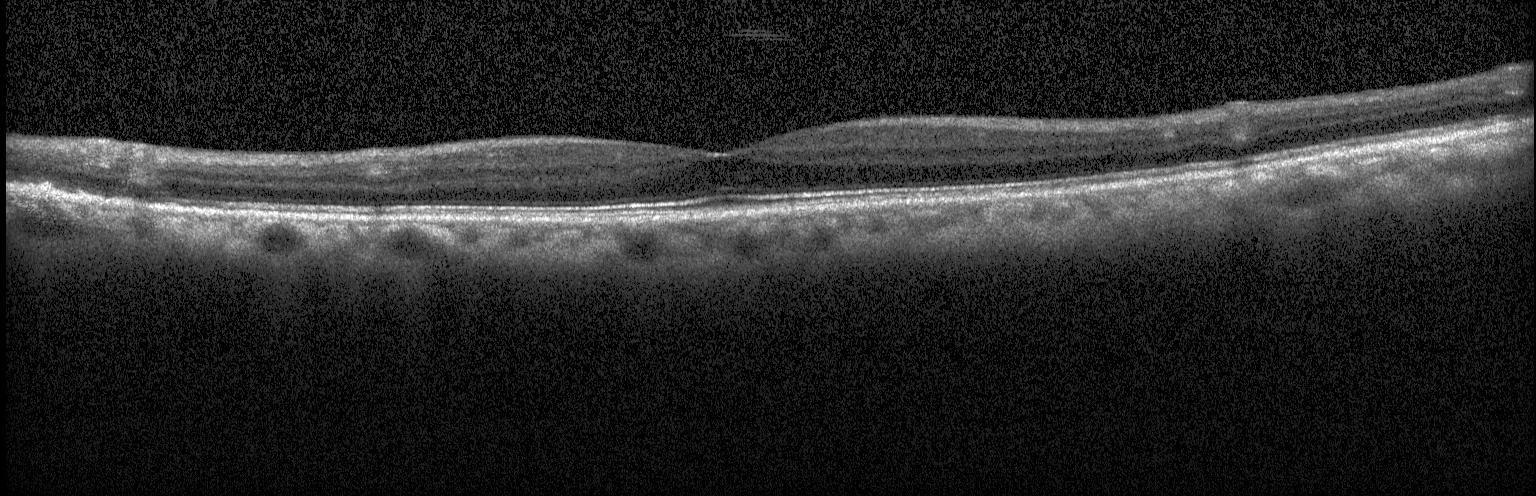
Optical coherence tomography scan — This B-scan demonstrates neither CNV, DME, nor drusen.